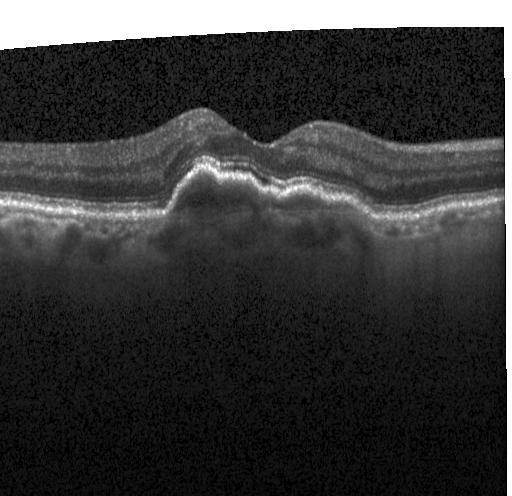
Finding: CNV.